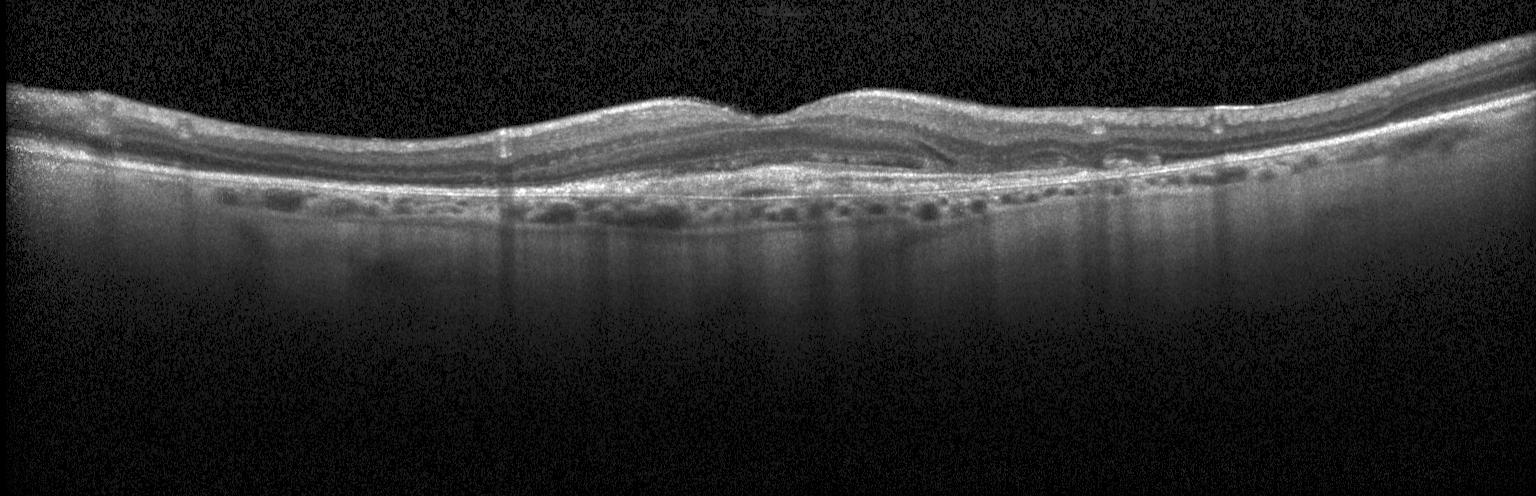
The scan shows a choroidal neovascular membrane.